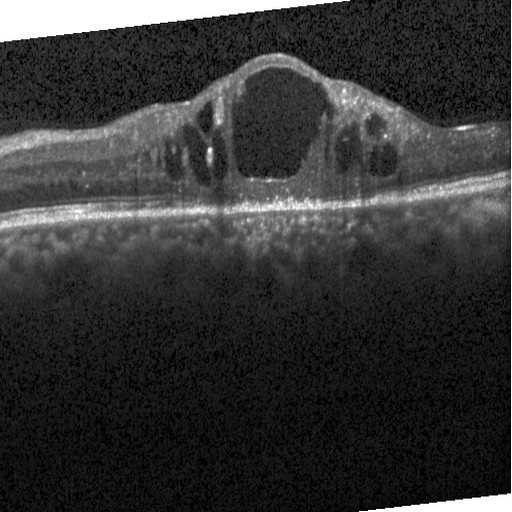

OCT line scan. OCT finding: DME.